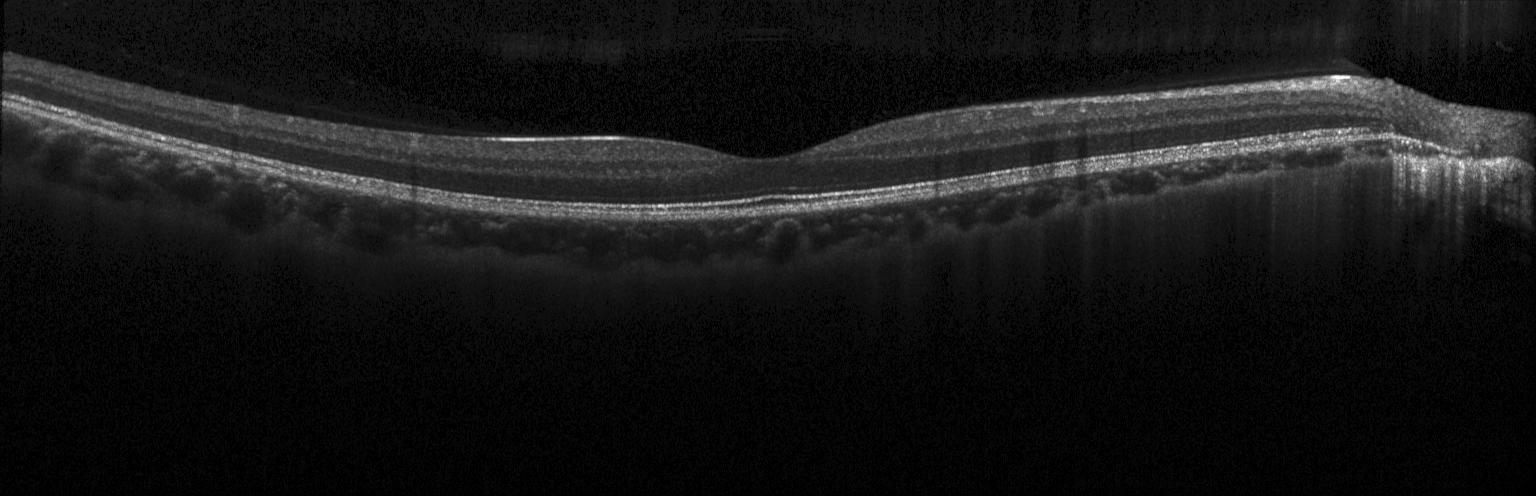
Retinal OCT cross-section — No choroidal neovascularization, no diabetic macular edema, and no drusen.